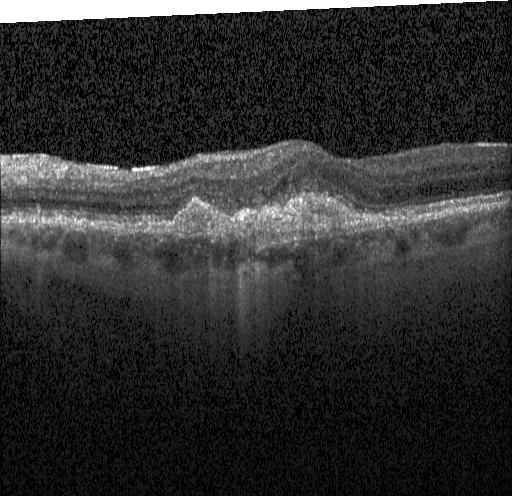

OCT line scan; fovea-centered
This B-scan demonstrates choroidal neovascularization (CNV).